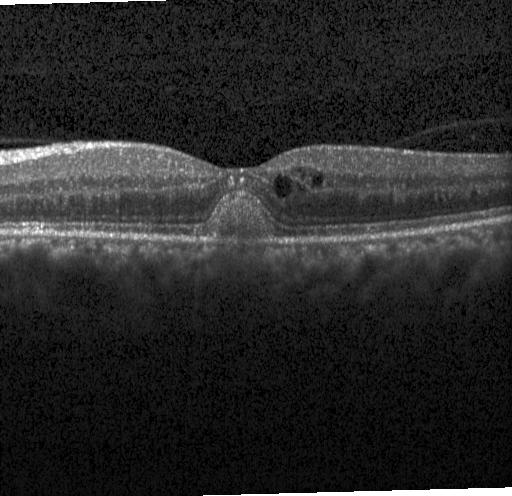

OCT B-scan showing a choroidal neovascular membrane.